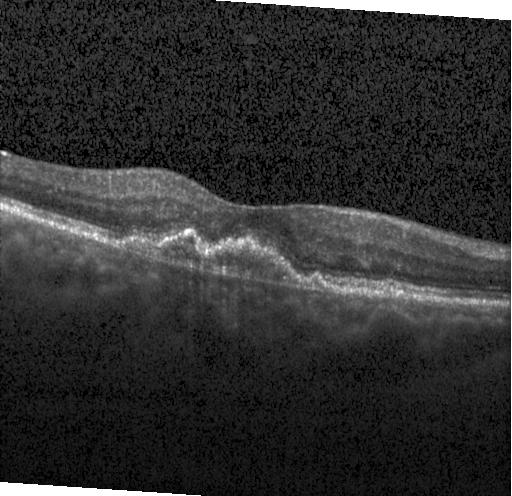
Dx: CNV.